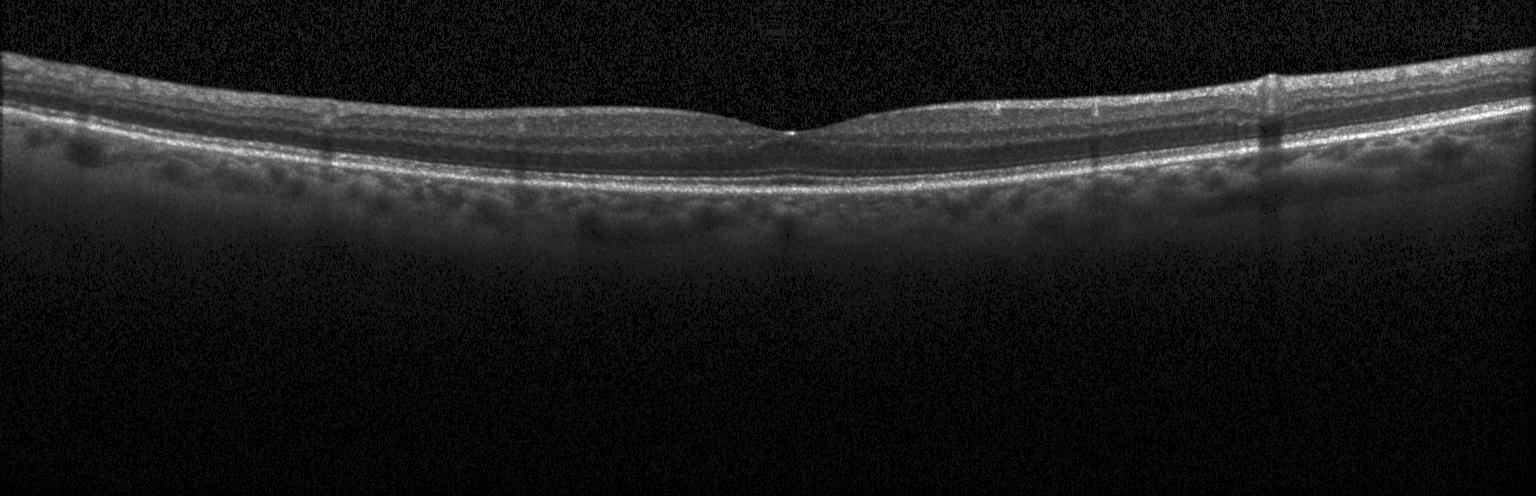
Diagnosis: no choroidal neovascularization, diabetic macular edema, or drusen.